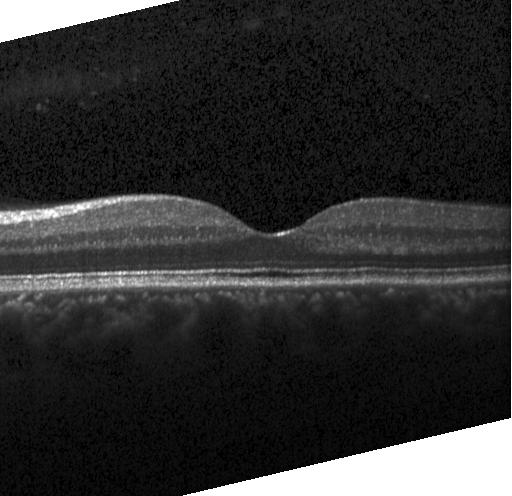
Instrument: Heidelberg Spectralis. Spectral-domain optical coherence tomography. Optical coherence tomography B-scan.
Impression: neither CNV, DME, nor drusen.